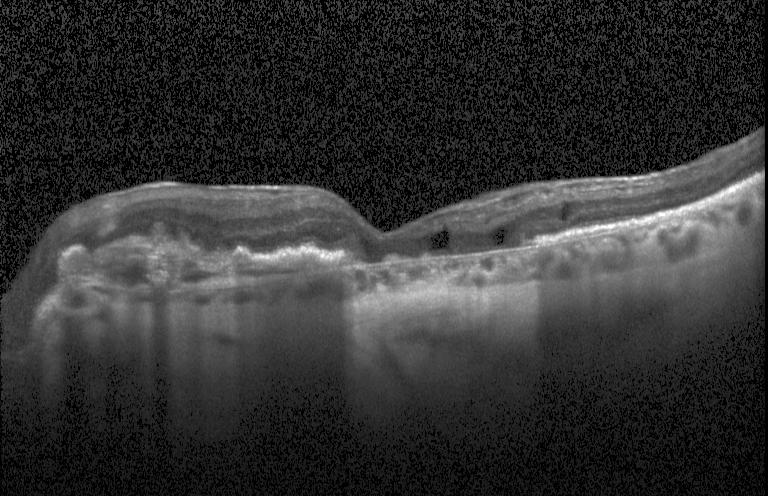 Optical coherence tomography scan.
The scan shows choroidal neovascularization.